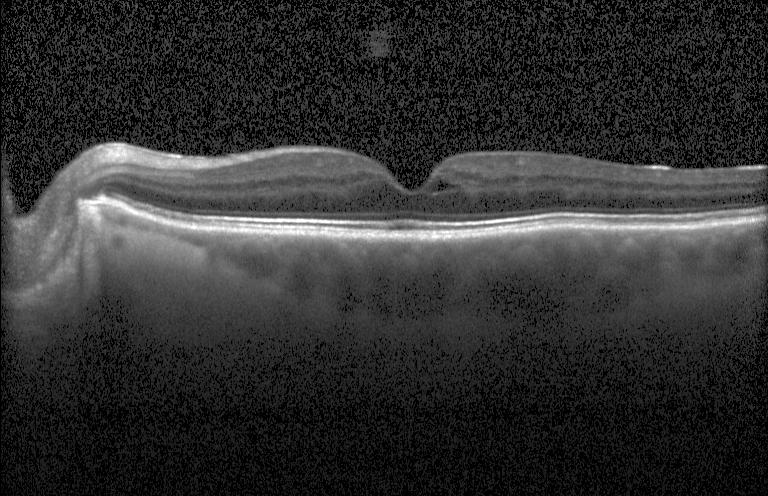 Heidelberg Spectralis OCT system, retinal OCT cross-section
This B-scan demonstrates diabetic macular edema (DME).